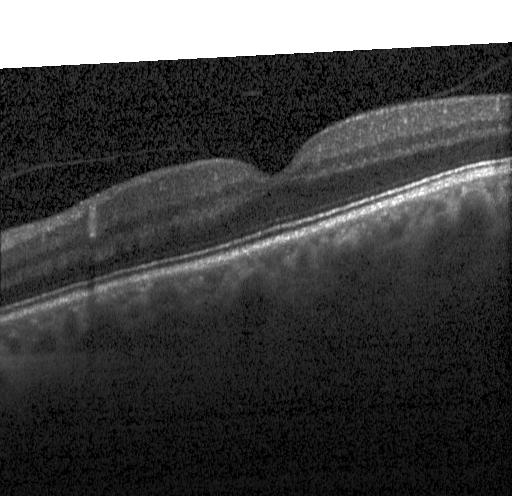 The scan shows no CNV, no DME, and no drusen.